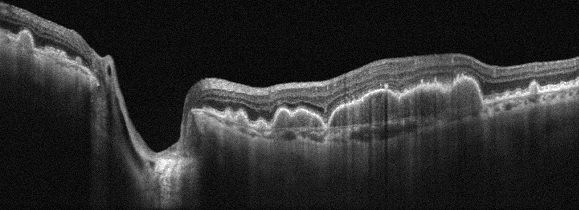 Diagnosis: age-related macular degeneration (AMD).